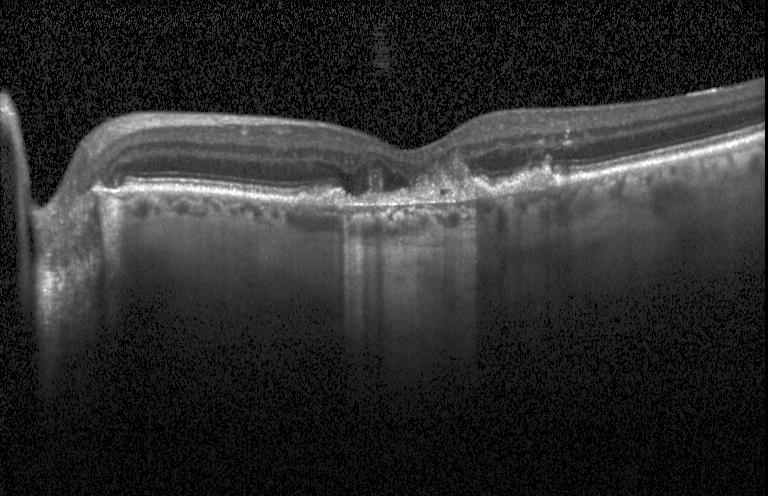
Optical coherence tomography scan — Assessment: CNV.